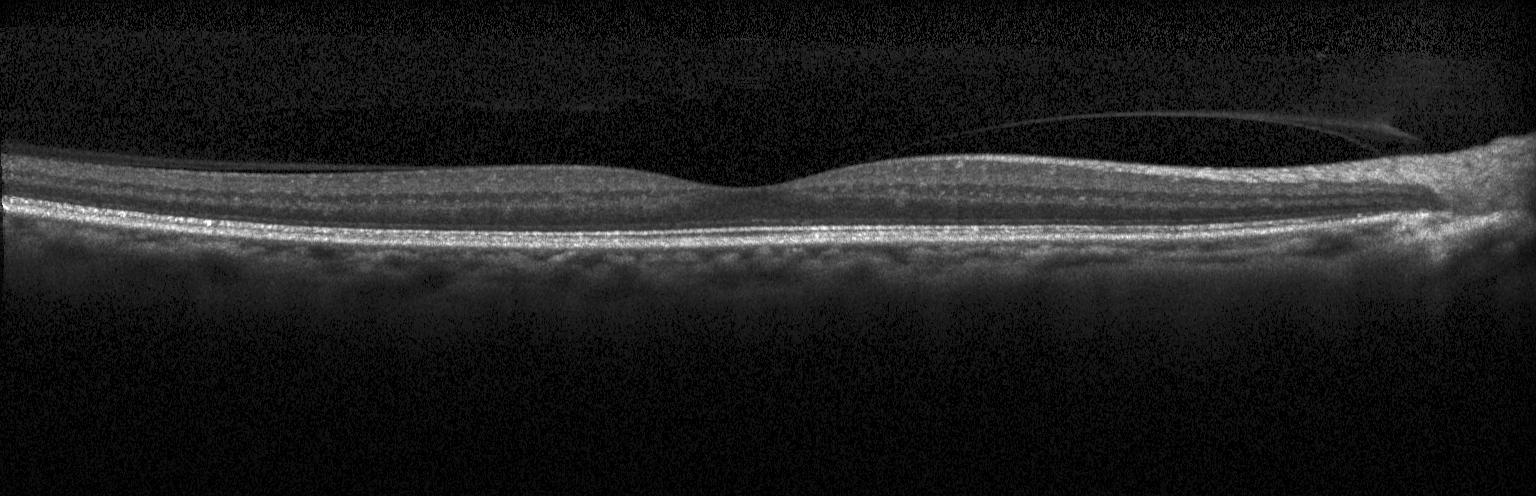 OCT B-scan. SD-OCT. Fovea-centered. Heidelberg Spectralis. Finding: no choroidal neovascularization, no diabetic macular edema, and no drusen.